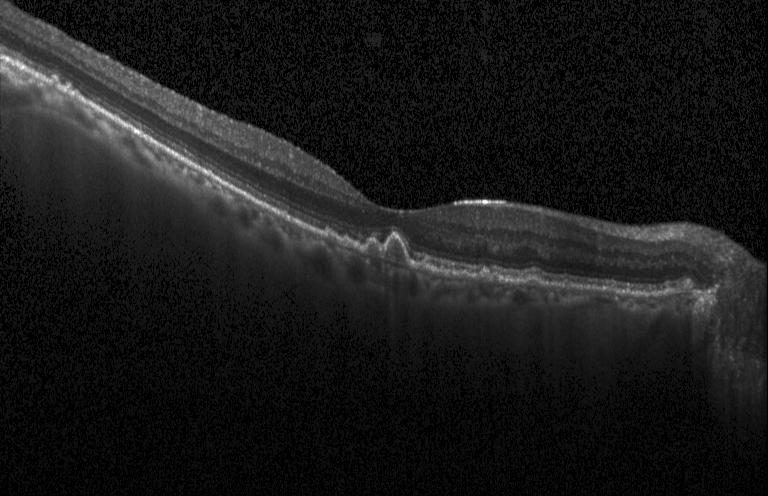

OCT B-scan
Impression: drusen.